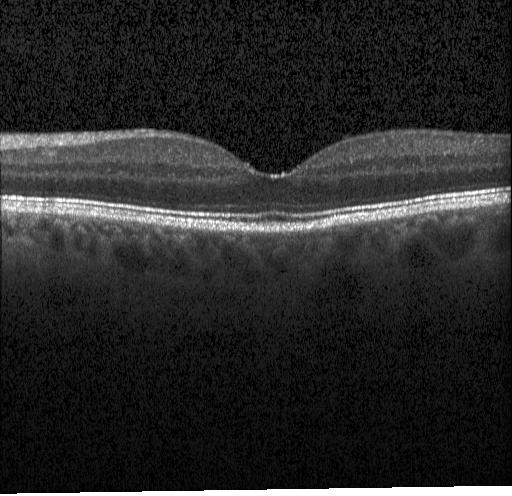

Diagnosis: no evidence of choroidal neovascularization, diabetic macular edema, or drusen.